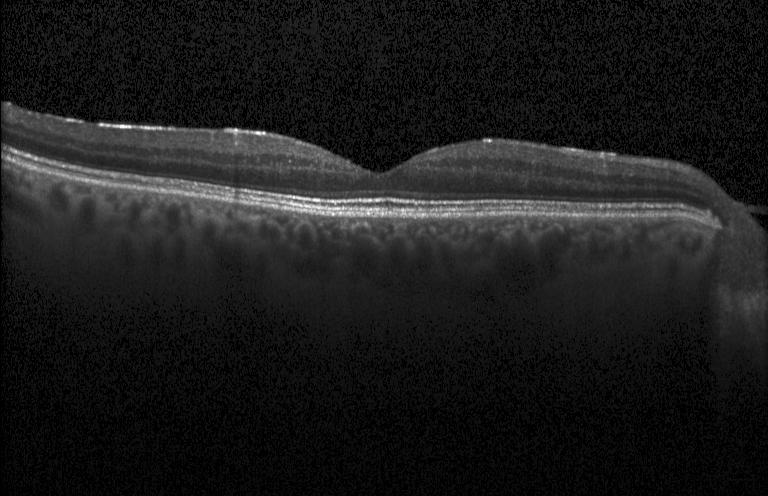

Optical coherence tomography B-scan. Assessment: neither CNV, DME, nor drusen.